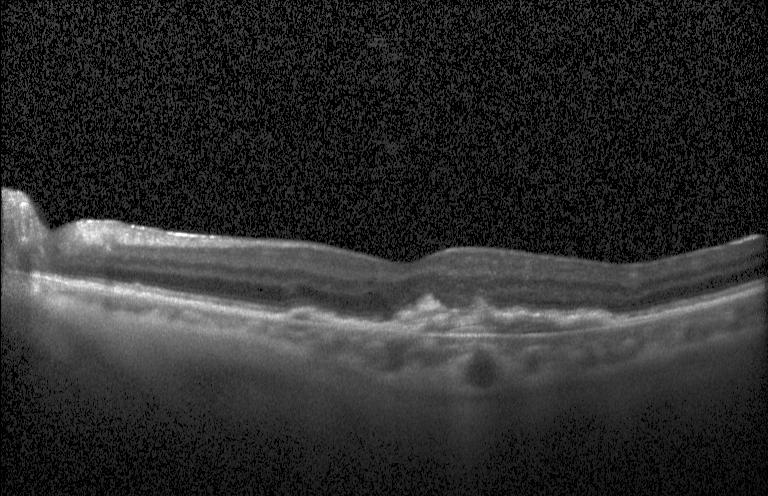

OCT finding: a choroidal neovascular membrane.